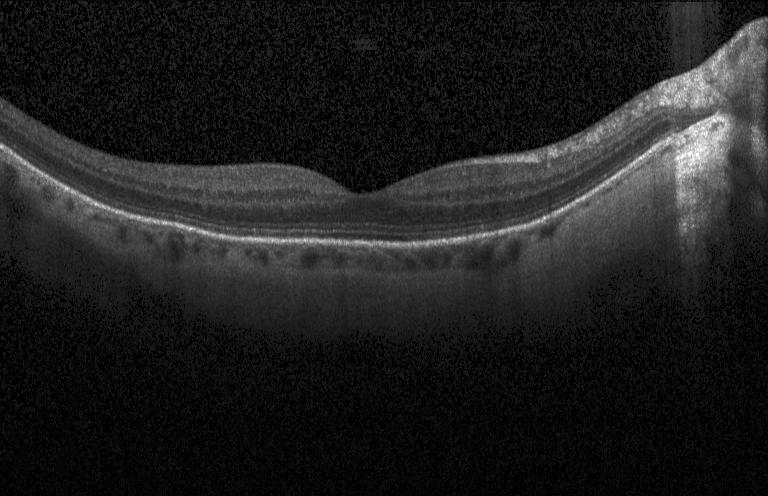
Retinal OCT cross-section. Spectral-domain optical coherence tomography. Instrument: Heidelberg Spectralis. Horizontal scan through the fovea.
Impression: no evidence of choroidal neovascularization, diabetic macular edema, or drusen.